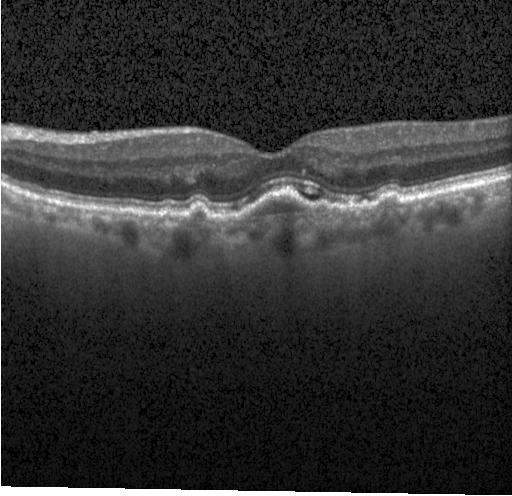 Optical coherence tomography B-scan, spectral-domain OCT, acquired on a Heidelberg Spectralis, macular scan
This B-scan demonstrates a choroidal neovascular membrane.